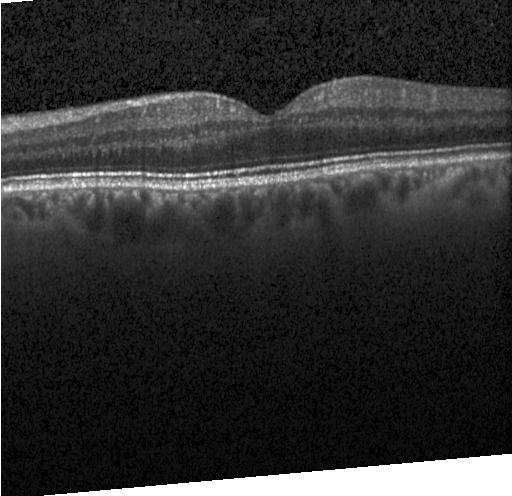 Retinal OCT cross-section. OCT finding: no CNV, no DME, and no drusen.